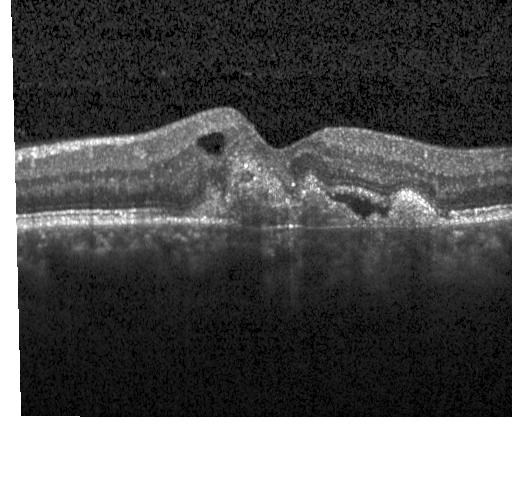

Retinal OCT cross-section. Instrument: Heidelberg Spectralis. Assessment: CNV.